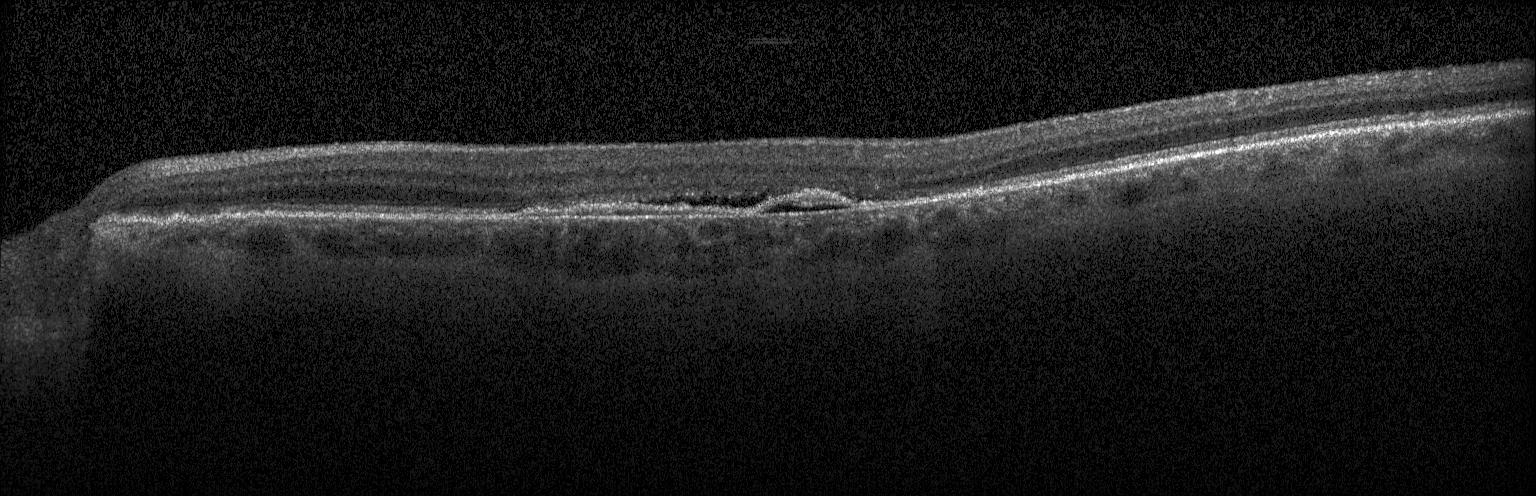 Retinal OCT B-scan.
Finding: a choroidal neovascular membrane.